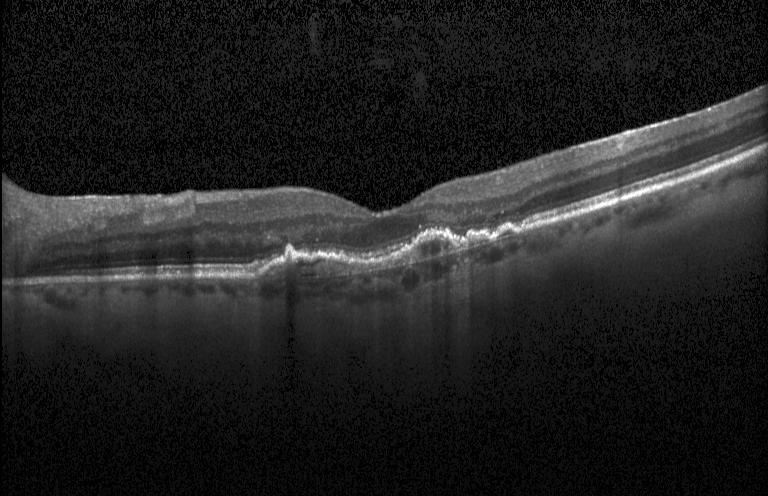
Through the macula; OCT line scan; instrument: Heidelberg Spectralis; spectral-domain optical coherence tomography — Finding: CNV.